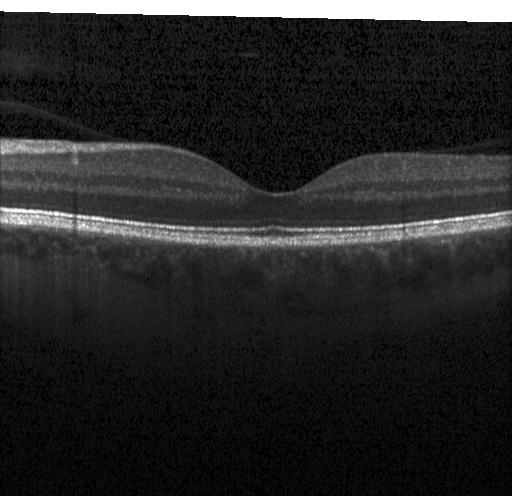 Diagnosis: no choroidal neovascularization, no diabetic macular edema, and no drusen.